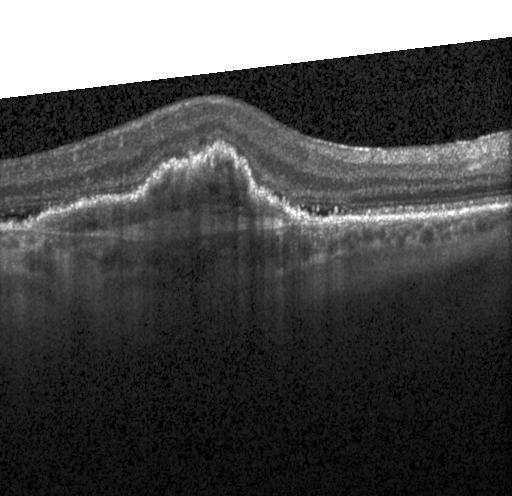
Optical coherence tomography B-scan.
Dx: choroidal neovascularization.